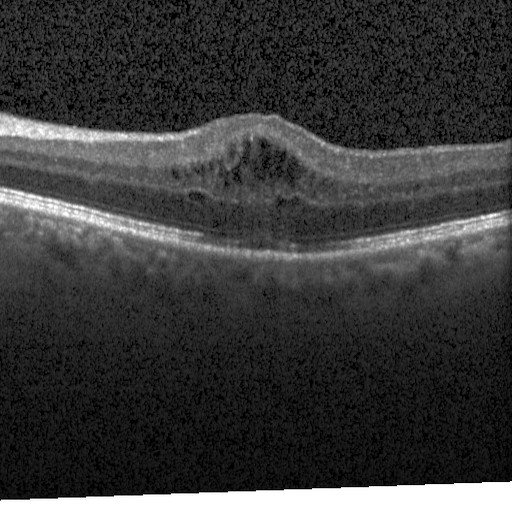
Retinal OCT B-scan, spectral-domain OCT — Finding: DME.